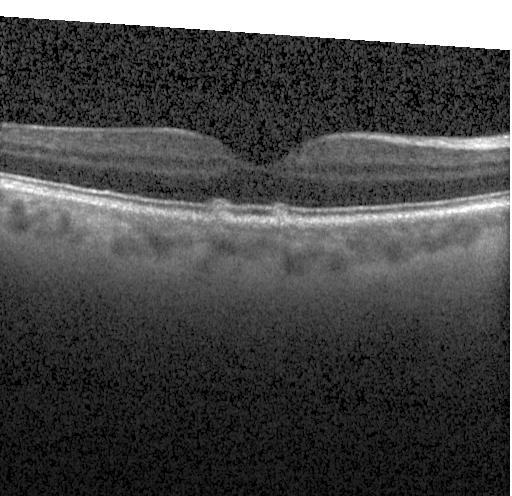

Spectral-domain OCT. Heidelberg Spectralis. OCT B-scan. Horizontal scan through the fovea. Impression: sub-RPE drusenoid deposits.